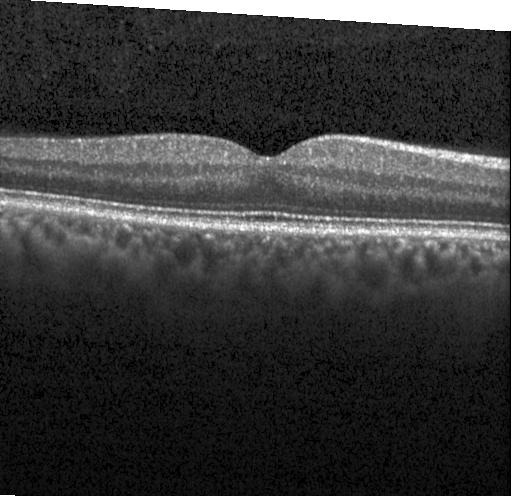

Acquired on a Heidelberg Spectralis · spectral-domain OCT · retinal OCT B-scan — Dx: neither choroidal neovascularization, diabetic macular edema, nor drusen.